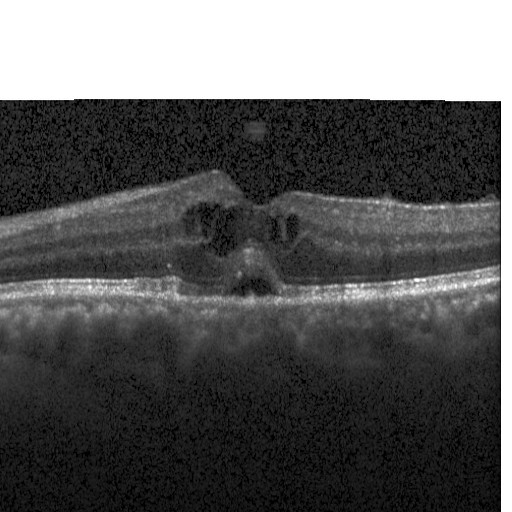
DME.